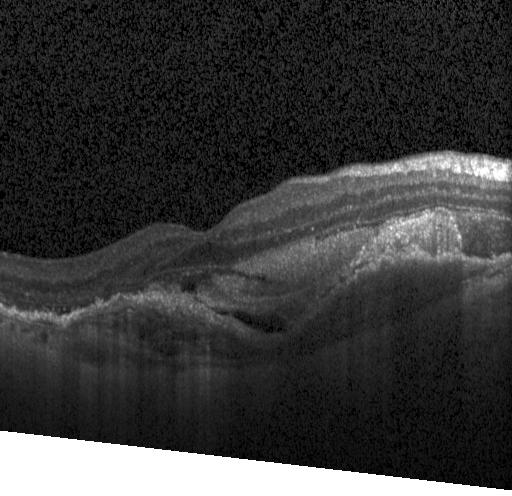
OCT line scan. Choroidal neovascularization (CNV).